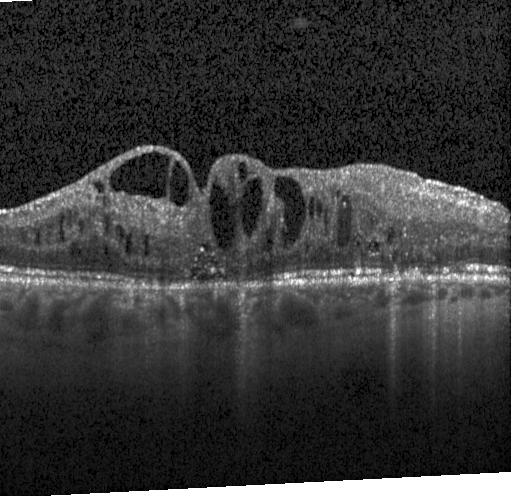
OCT B-scan; SD-OCT
Dx: diabetic macular edema (DME).